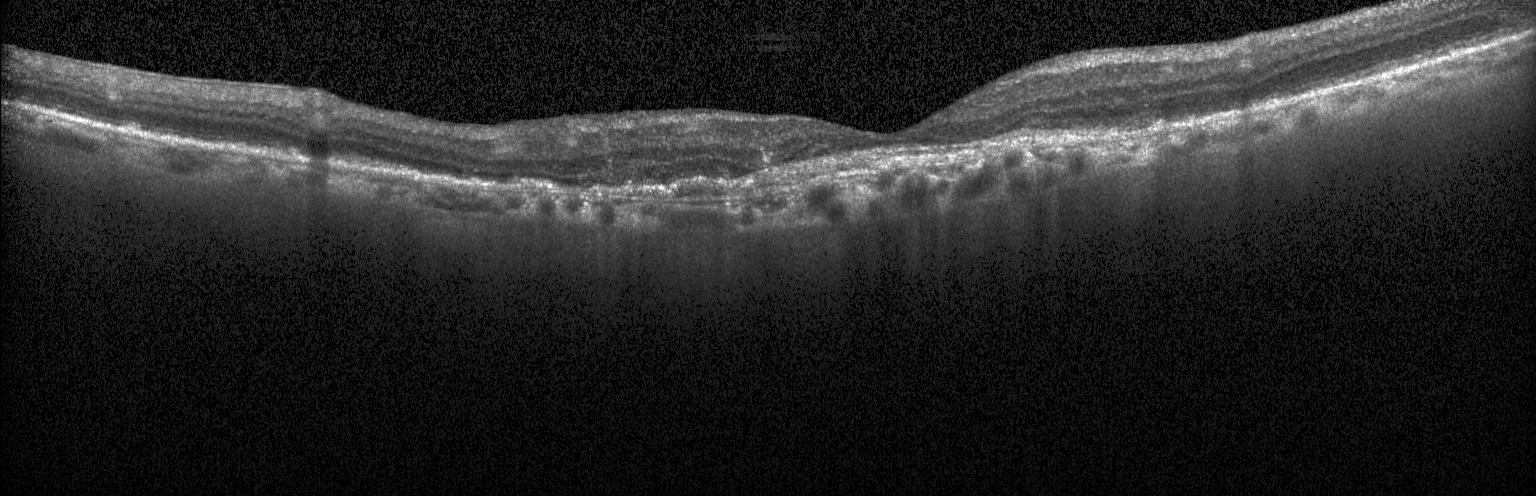

Instrument: Heidelberg Spectralis. SD-OCT. Horizontal scan through the fovea. OCT B-scan — Finding: a choroidal neovascular membrane.